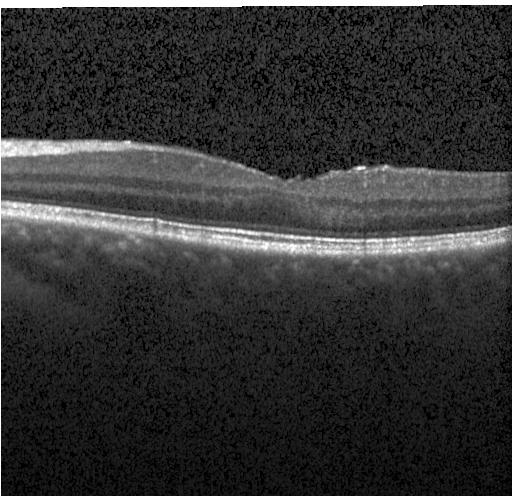 Spectral-domain optical coherence tomography, OCT line scan, Heidelberg Spectralis, through the macula.
Diagnosis: no choroidal neovascularization, diabetic macular edema, or drusen.